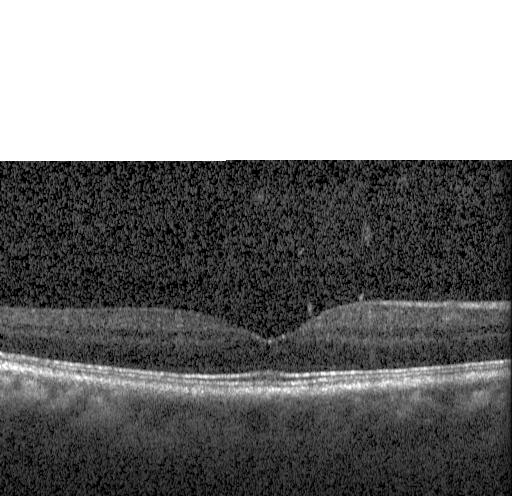
Optical coherence tomography scan. Spectral-domain OCT. Fovea-centered. Heidelberg Spectralis OCT system
OCT finding: no choroidal neovascularization, no diabetic macular edema, and no drusen.